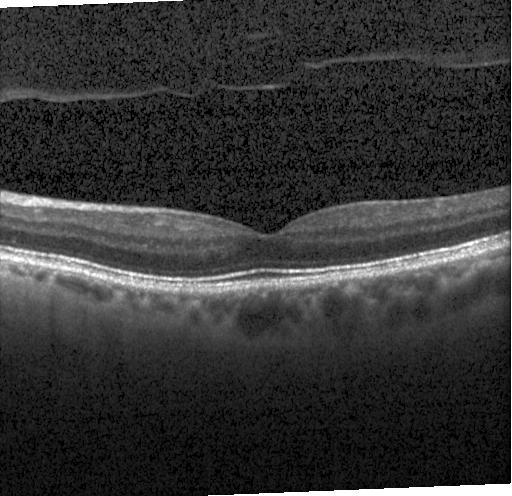
OCT B-scan — Impression: no evidence of CNV, DME, or drusen.